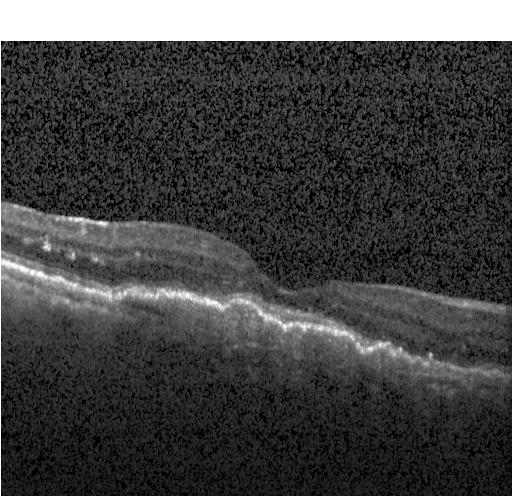 Spectral-domain OCT B-scan: a choroidal neovascular membrane.